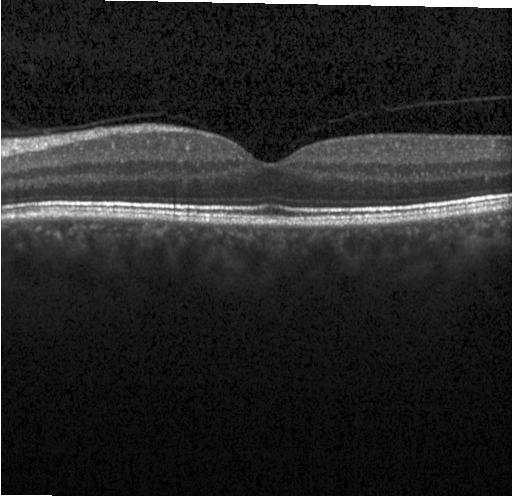 OCT scan showing no evidence of choroidal neovascularization, diabetic macular edema, or drusen.